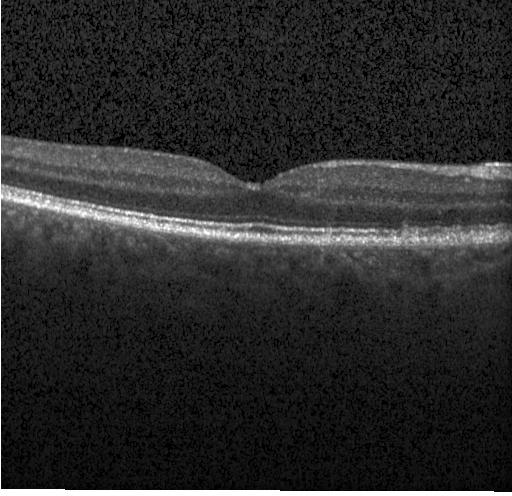
OCT B-scan
Finding: multiple drusen.